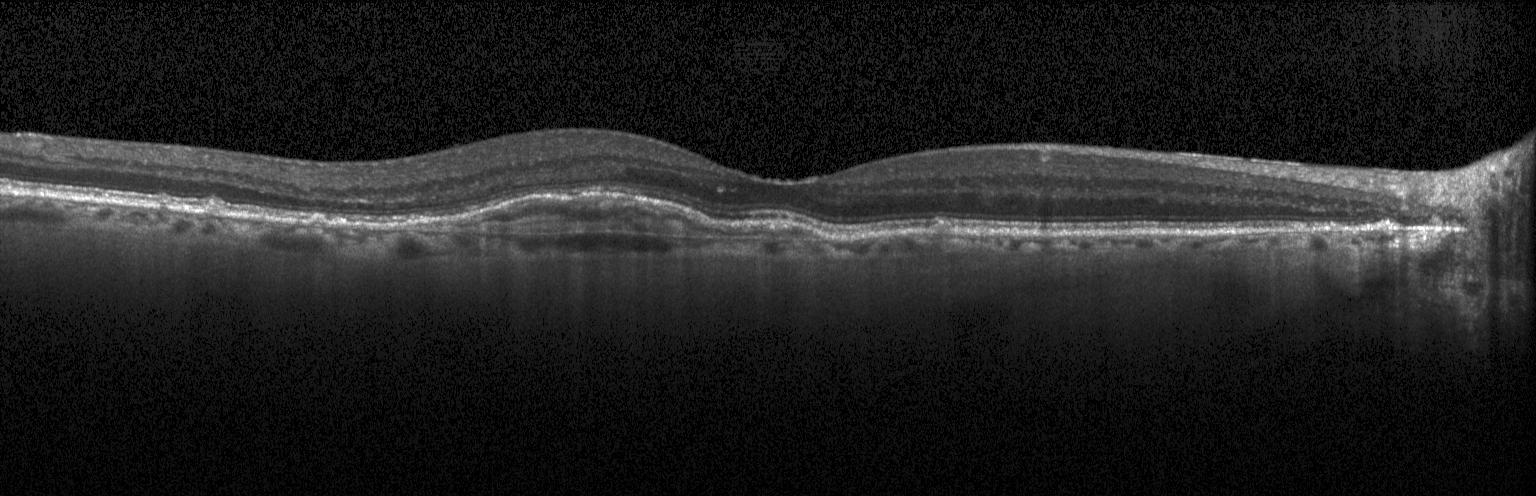
Finding: CNV.